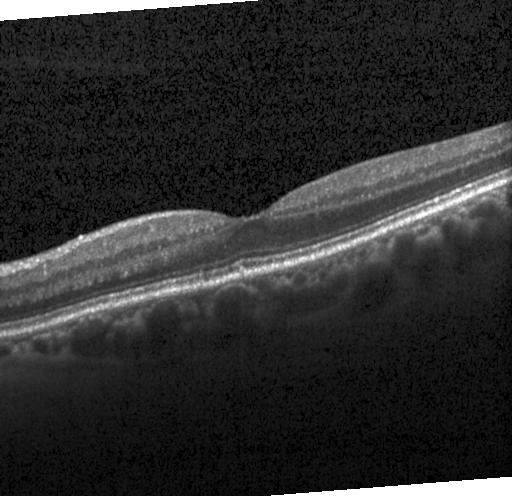

OCT scan showing no choroidal neovascularization, diabetic macular edema, or drusen.